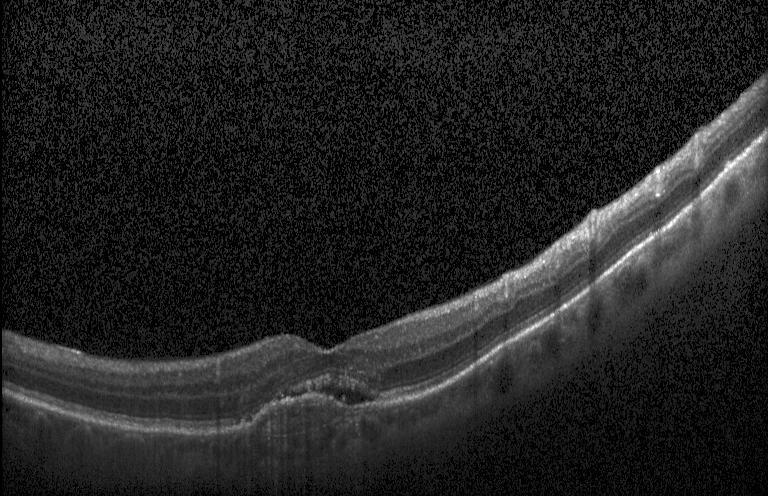

Finding: choroidal neovascularization.